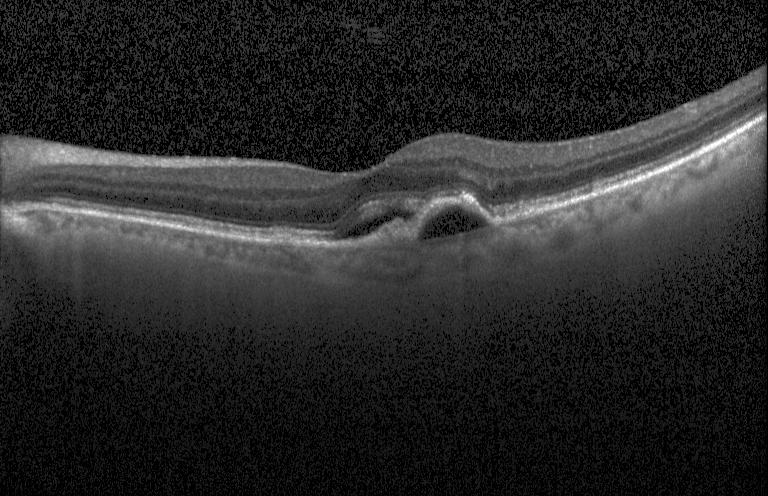

SD-OCT, macular scan, retinal OCT cross-section, Heidelberg Spectralis
The scan shows choroidal neovascularization.